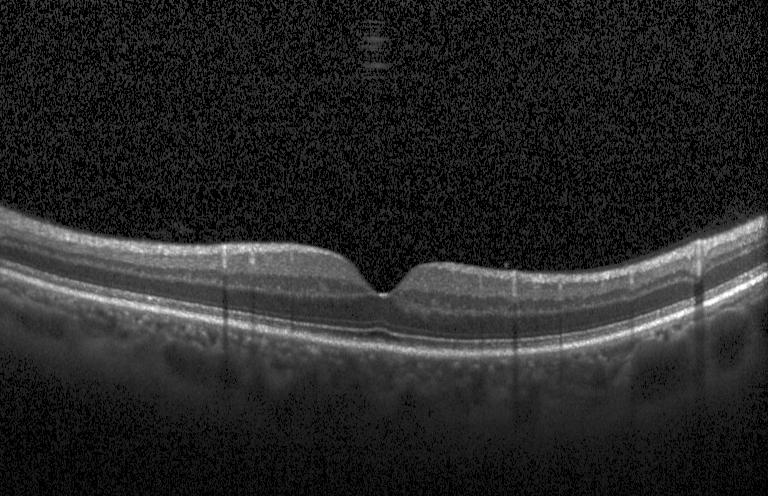

Spectral-domain OCT · optical coherence tomography B-scan · centered on the fovea · Heidelberg Spectralis — Finding: no choroidal neovascularization, no diabetic macular edema, and no drusen.